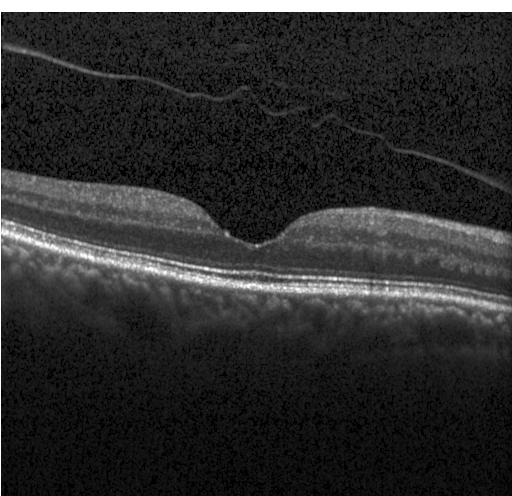

Retinal OCT B-scan.
Macular OCT: no evidence of CNV, DME, or drusen.